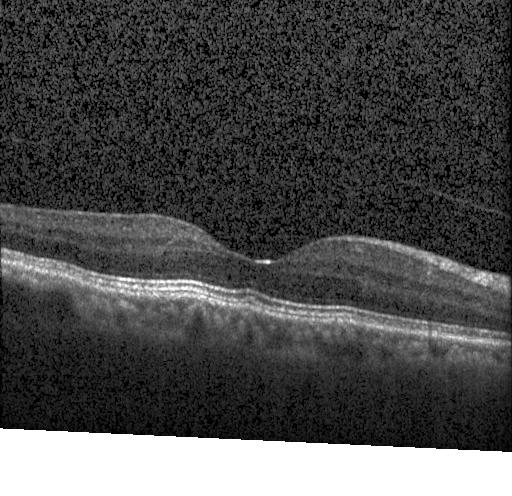

Impression: no choroidal neovascularization, no diabetic macular edema, and no drusen.